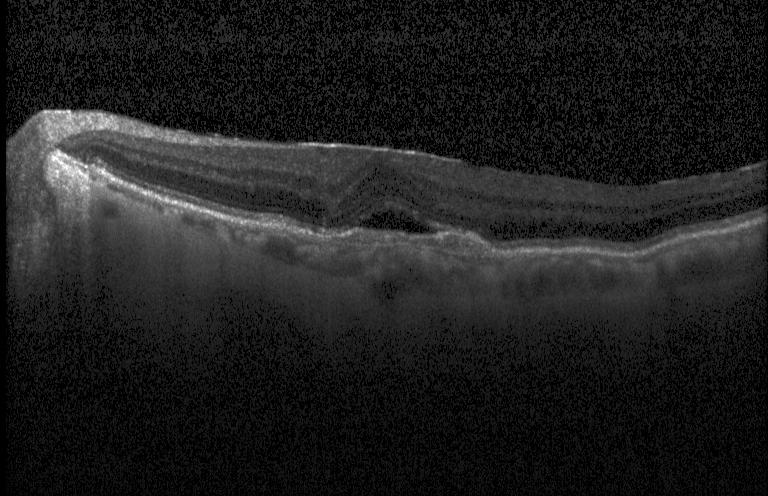

OCT B-scan
The scan shows a choroidal neovascular membrane.